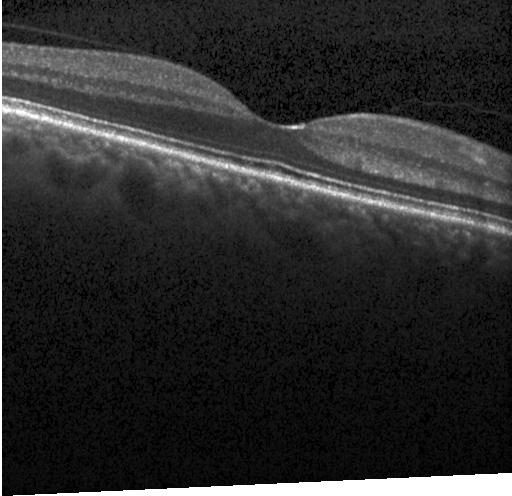
OCT B-scan showing no evidence of CNV, DME, or drusen.